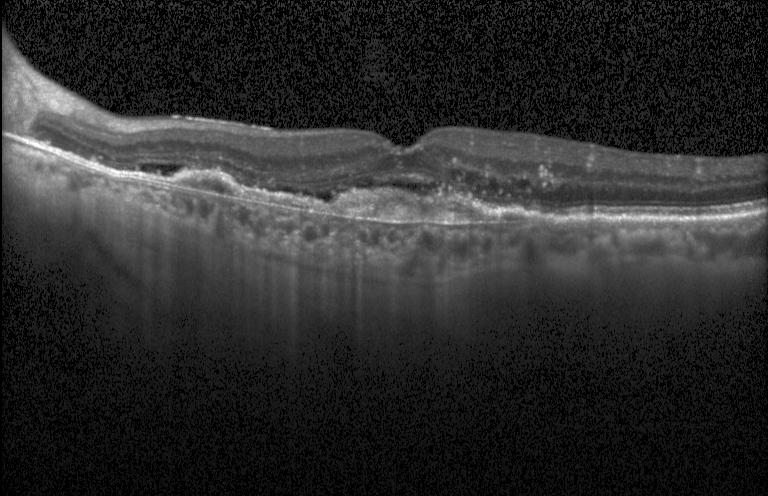

The scan shows CNV.